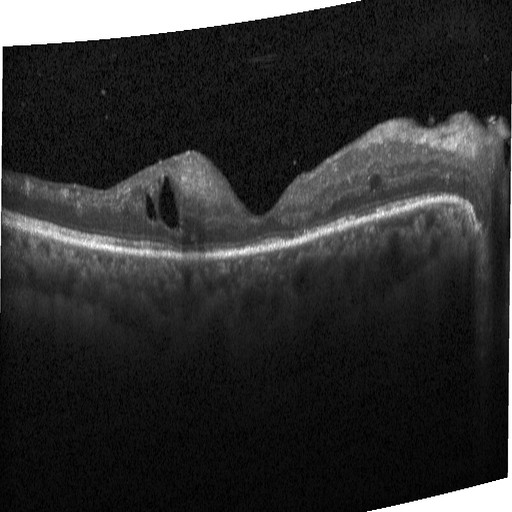
Spectral-domain optical coherence tomography · OCT B-scan. Finding: diabetic macular edema.